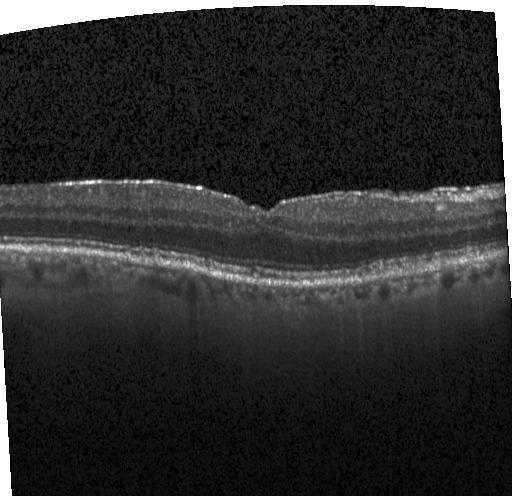 OCT line scan. Impression: multiple drusen.